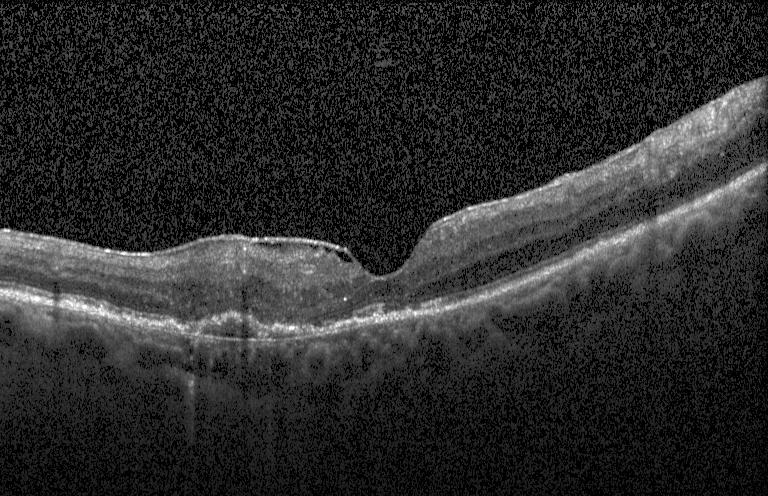 Heidelberg Spectralis · through the macula · SD-OCT · retinal OCT B-scan — The scan shows choroidal neovascularization (CNV).